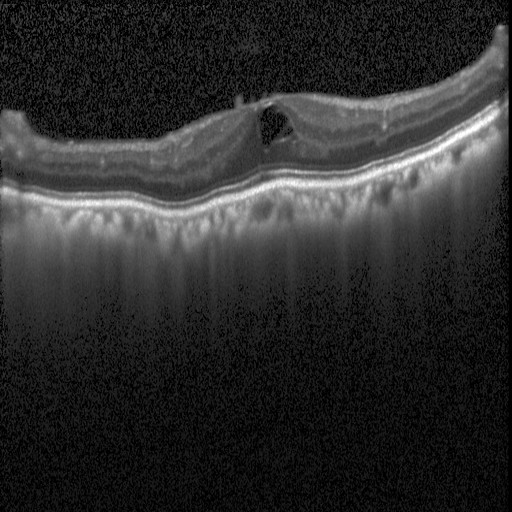
OCT scan showing diabetic macular edema (DME).